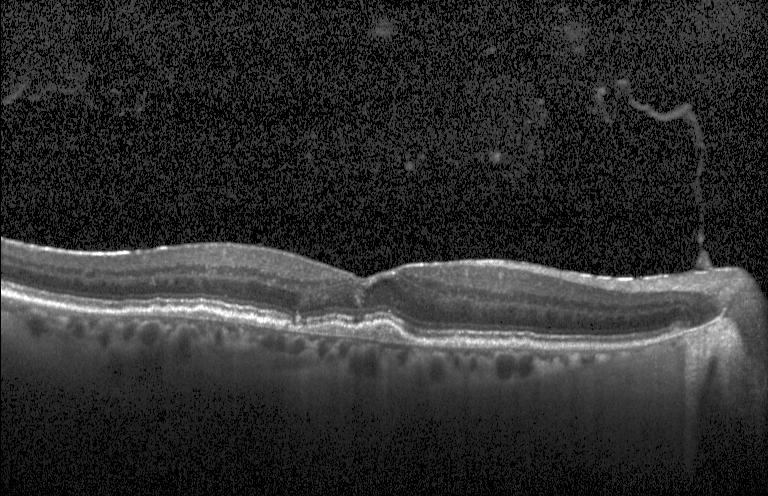 Instrument: Heidelberg Spectralis; retinal OCT B-scan; spectral-domain OCT — Macular OCT: choroidal neovascularization.